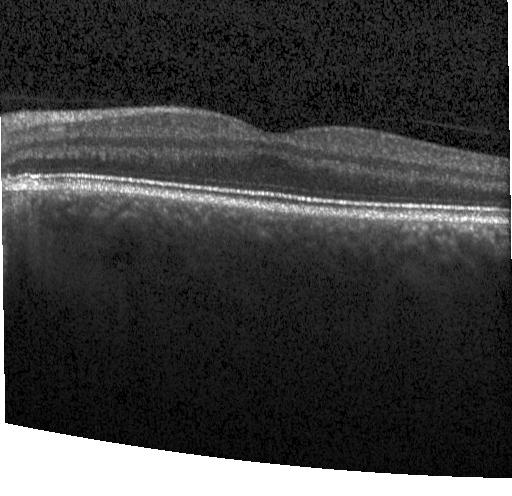 Spectral-domain optical coherence tomography, fovea-centered, Heidelberg Spectralis OCT system, optical coherence tomography B-scan
Finding: no CNV, no DME, and no drusen.